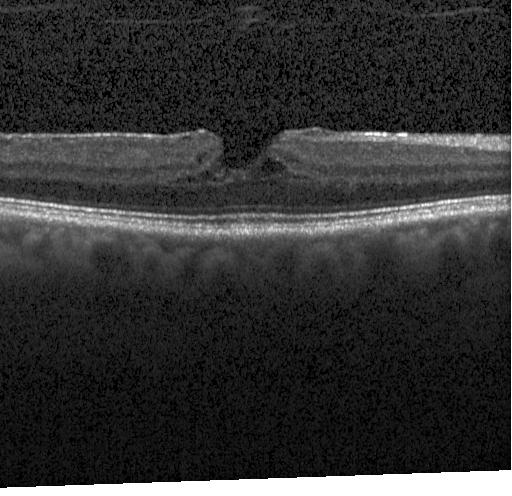

Finding: DME.